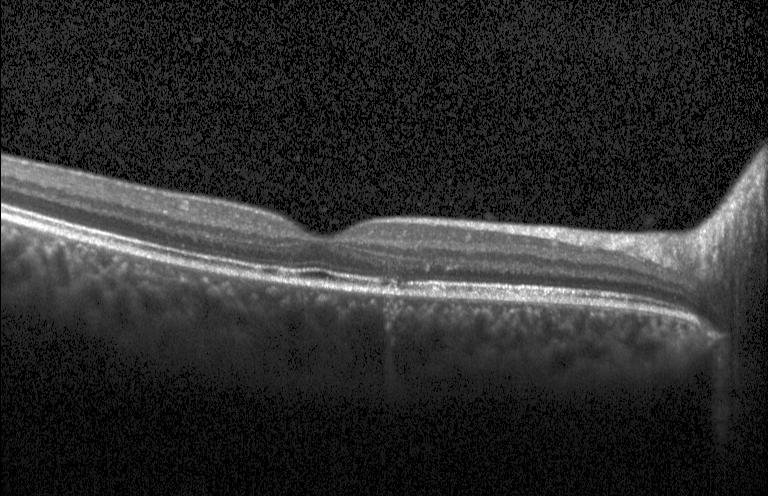 Diagnosis: multiple drusen.